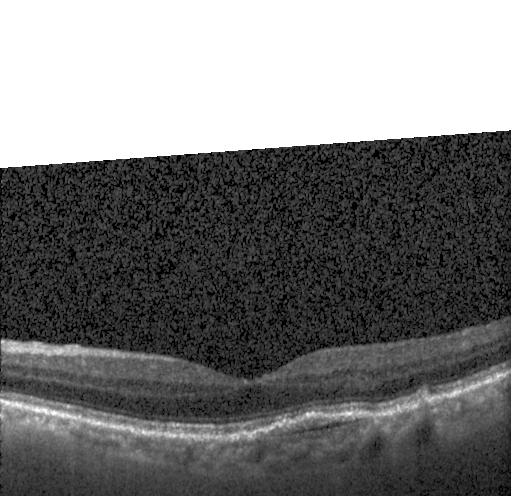

Macular scan, OCT B-scan, spectral-domain optical coherence tomography — This B-scan demonstrates choroidal neovascularization (CNV).